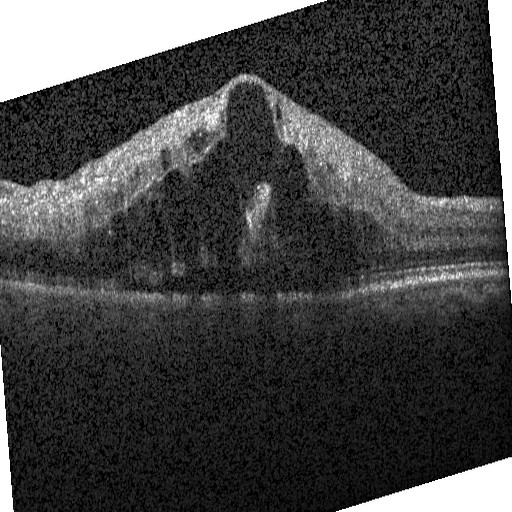 Horizontal scan through the fovea; spectral-domain optical coherence tomography; OCT B-scan; instrument: Heidelberg Spectralis — Dx: DME.